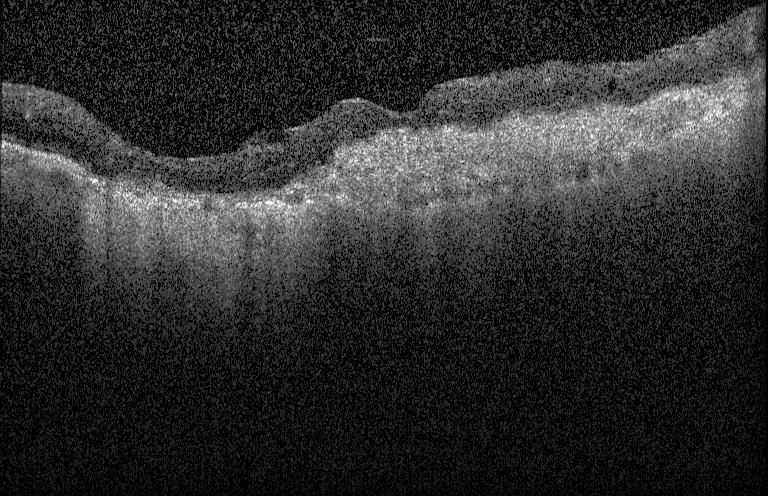
OCT scan showing choroidal neovascularization (CNV).